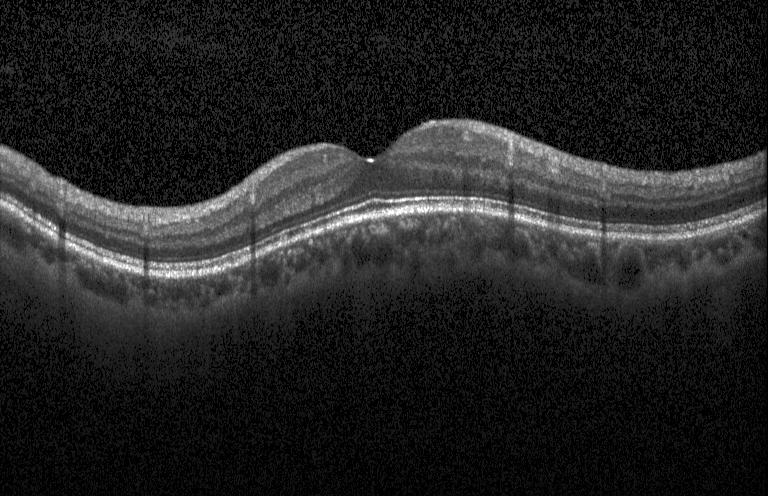
Impression: no choroidal neovascularization, no diabetic macular edema, and no drusen.